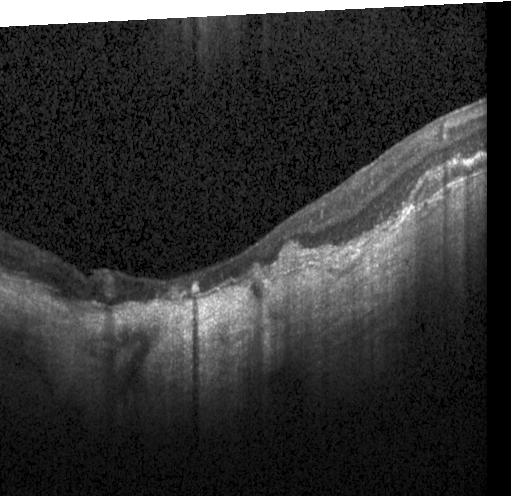
OCT B-scan. Heidelberg Spectralis OCT system. Spectral-domain optical coherence tomography. Through the macula
Diagnosis: choroidal neovascularization (CNV).